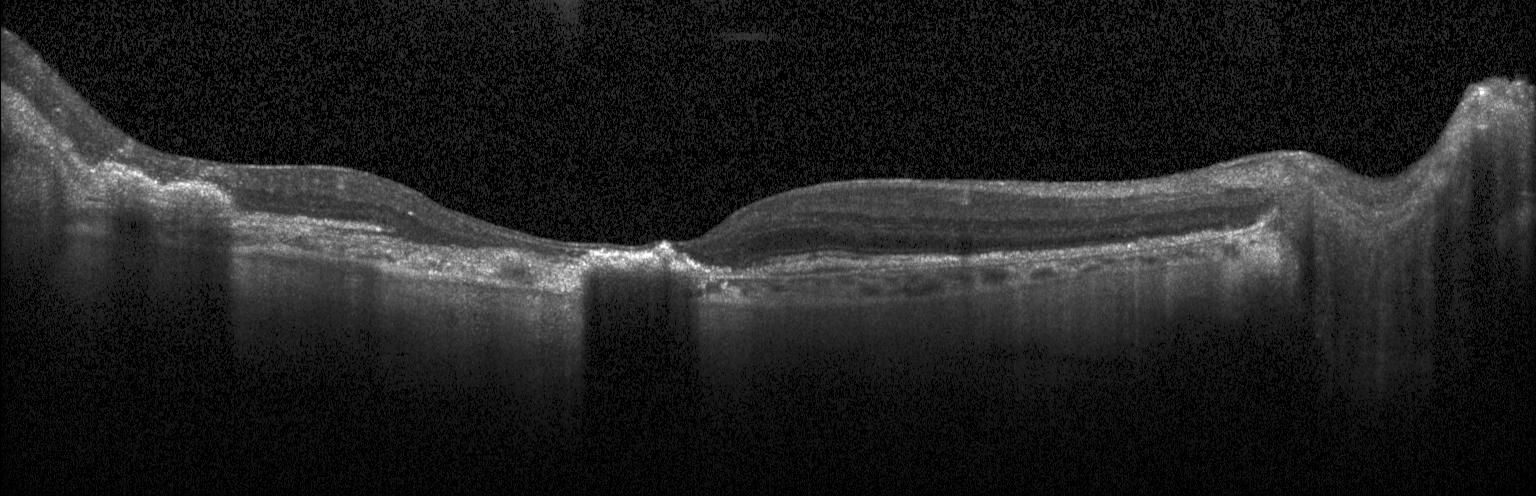 A choroidal neovascular membrane.